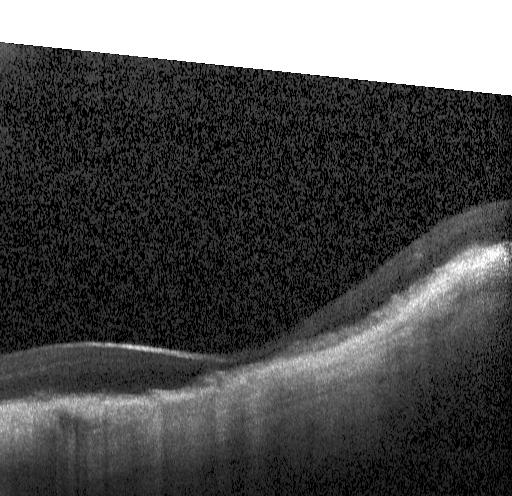
OCT line scan.
Macular OCT: a choroidal neovascular membrane.